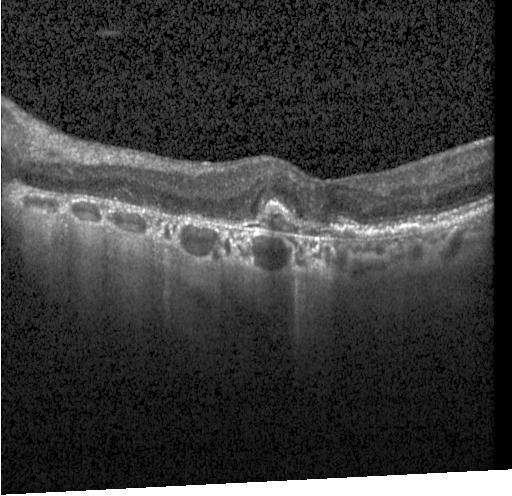
Instrument: Heidelberg Spectralis · spectral-domain OCT · optical coherence tomography B-scan · horizontal scan through the fovea.
Assessment: CNV.